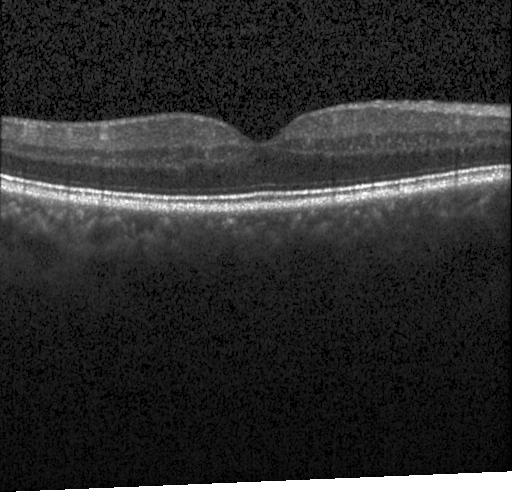
Spectral-domain optical coherence tomography. Horizontal scan through the fovea. OCT line scan. Heidelberg Spectralis. Dx: neither CNV, DME, nor drusen.